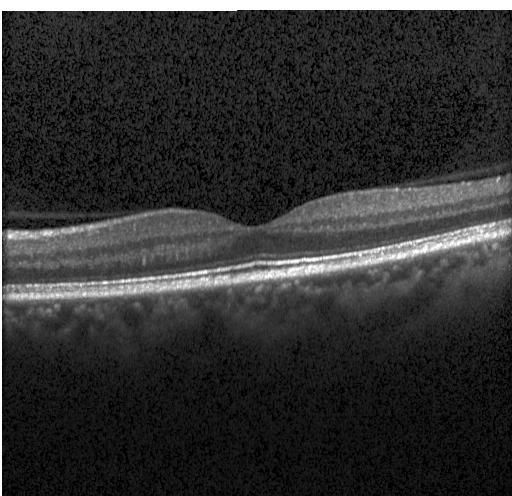
OCT line scan. The scan shows no CNV, no DME, and no drusen.